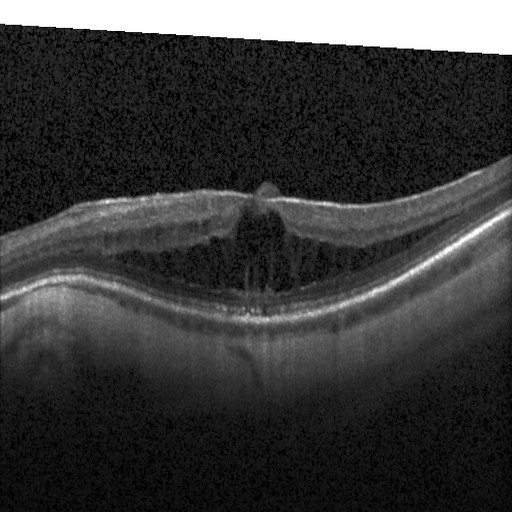 OCT B-scan; spectral-domain OCT; fovea-centered — Finding: diabetic macular edema (DME).